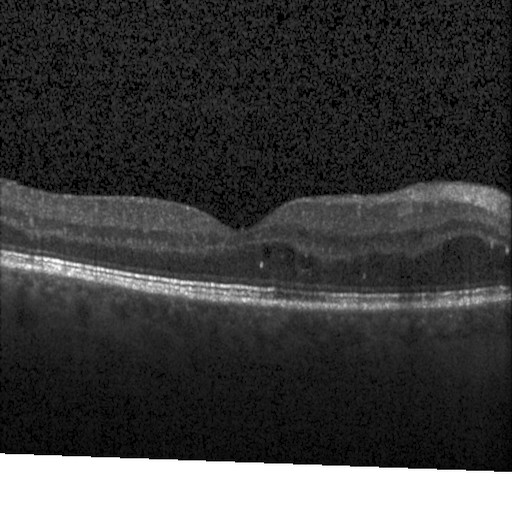

Optical coherence tomography B-scan.
Impression: diabetic macular edema (DME).